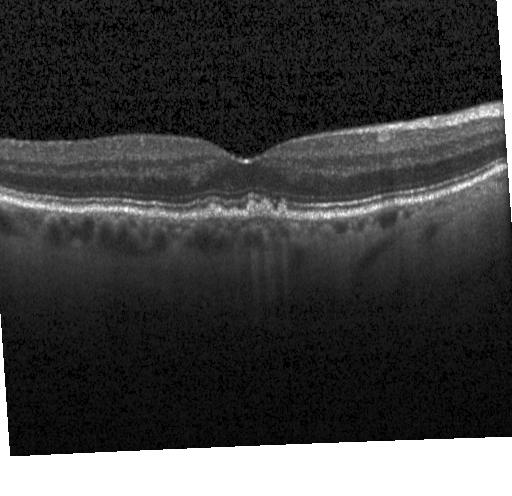
Impression: multiple drusen.